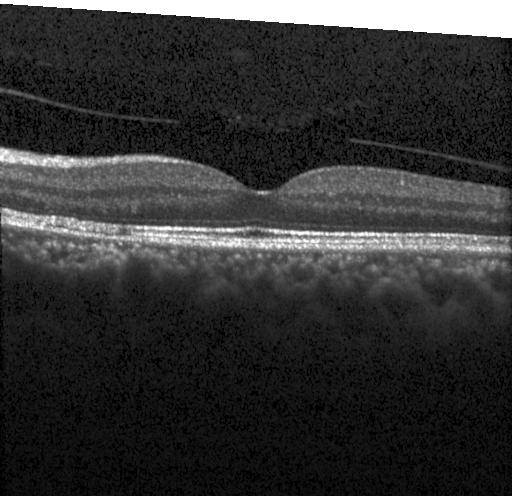

Diagnosis: no CNV, no DME, and no drusen.